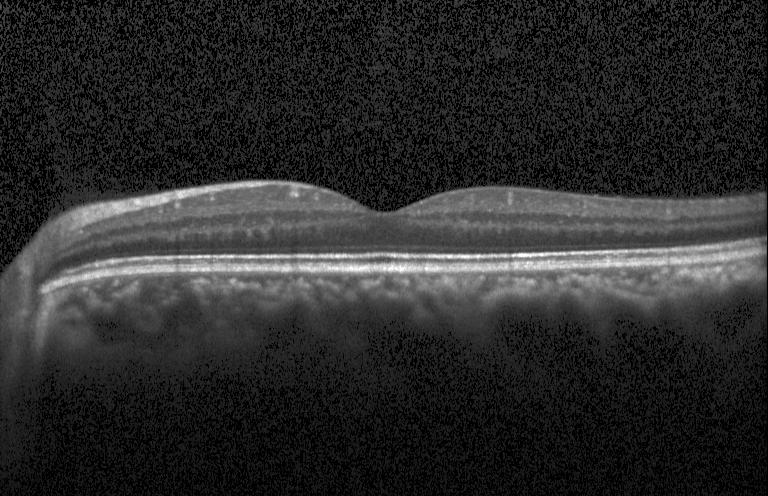 Finding: no evidence of CNV, DME, or drusen.